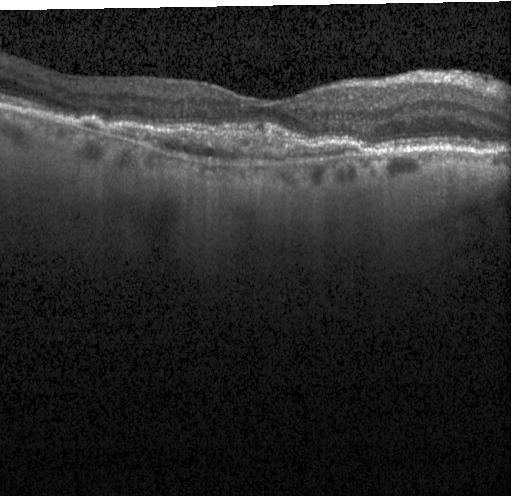 OCT B-scan showing a choroidal neovascular membrane.